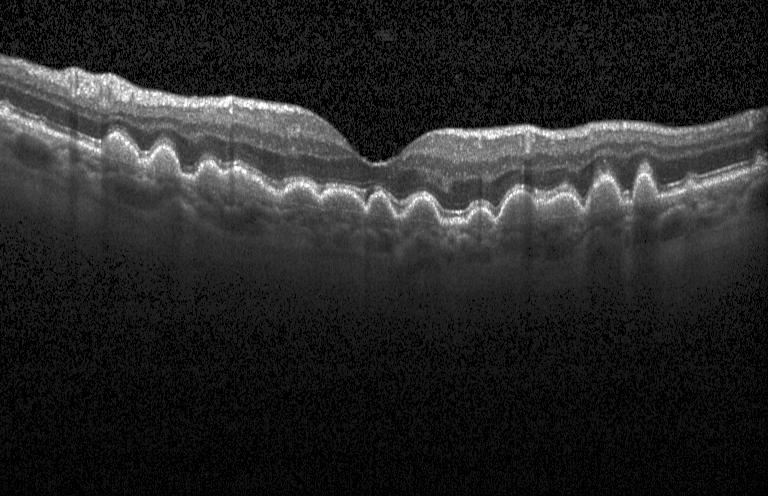 Retinal OCT B-scan. Acquired on a Heidelberg Spectralis. Centered on the fovea. Spectral-domain OCT.
Diagnosis: sub-RPE drusenoid deposits.